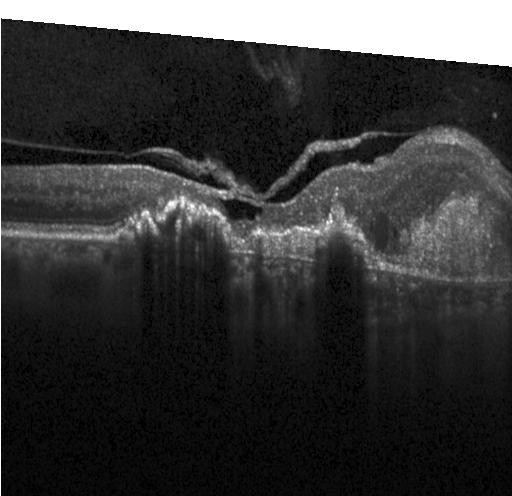
Spectral-domain OCT, optical coherence tomography scan, macular scan
Finding: a choroidal neovascular membrane.